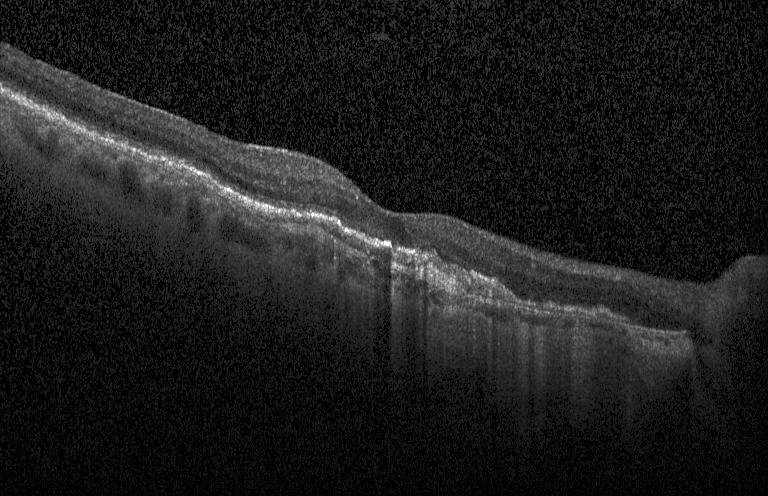

Optical coherence tomography scan; centered on the fovea; SD-OCT.
Finding: choroidal neovascularization.